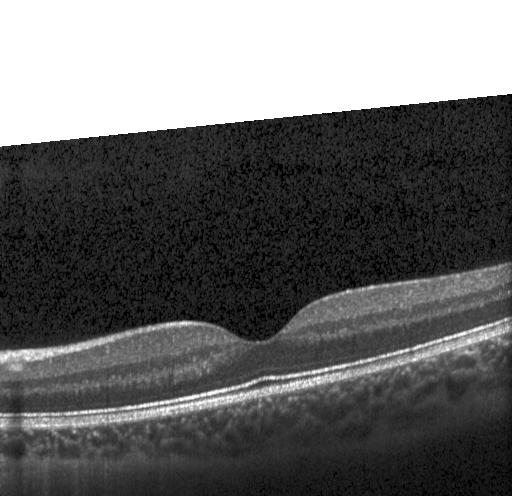 Spectral-domain optical coherence tomography, OCT B-scan.
Impression: no choroidal neovascularization, no diabetic macular edema, and no drusen.